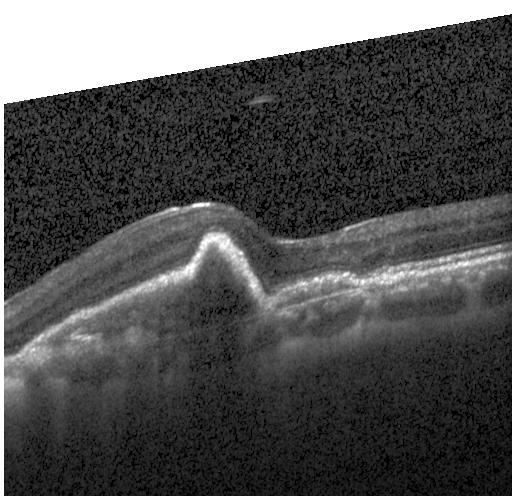

Spectral-domain OCT; OCT line scan; fovea-centered. This B-scan demonstrates choroidal neovascularization (CNV).